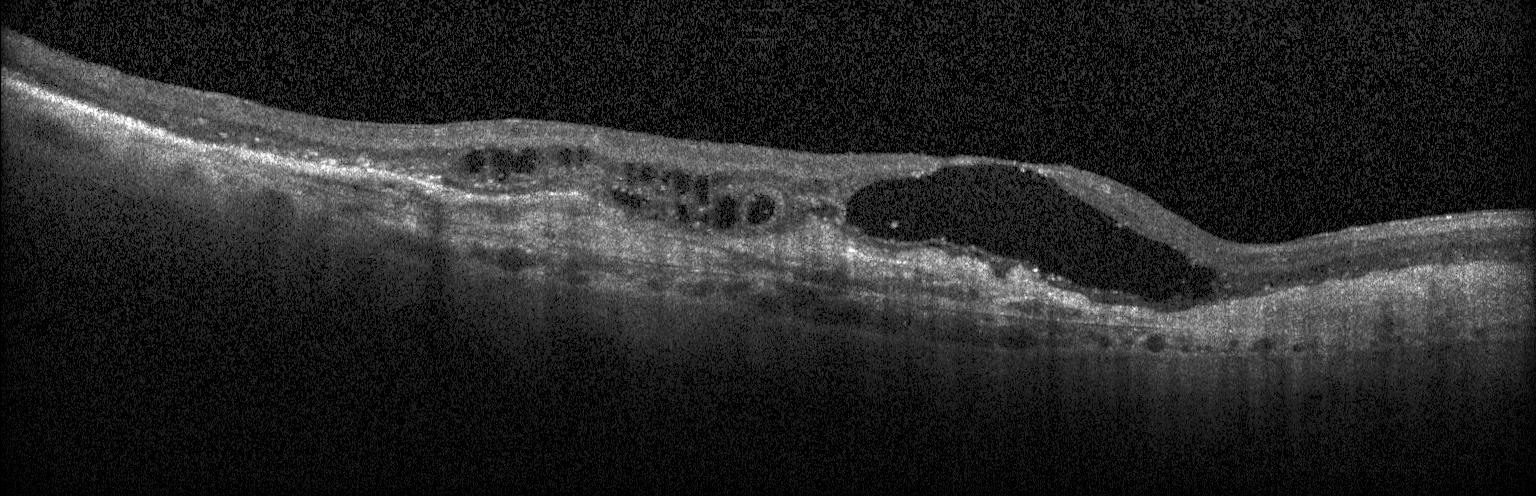 OCT line scan — This B-scan demonstrates a choroidal neovascular membrane.